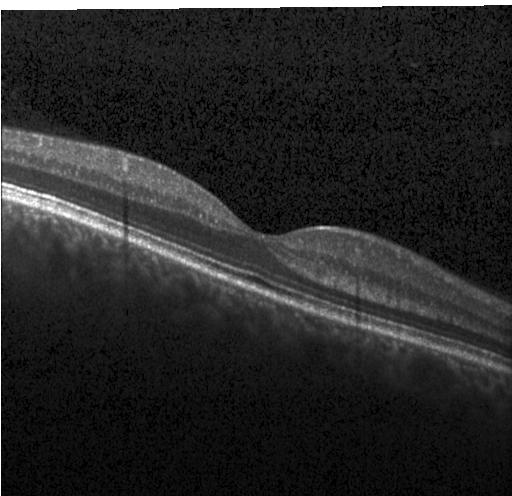 The scan shows no evidence of choroidal neovascularization, diabetic macular edema, or drusen.